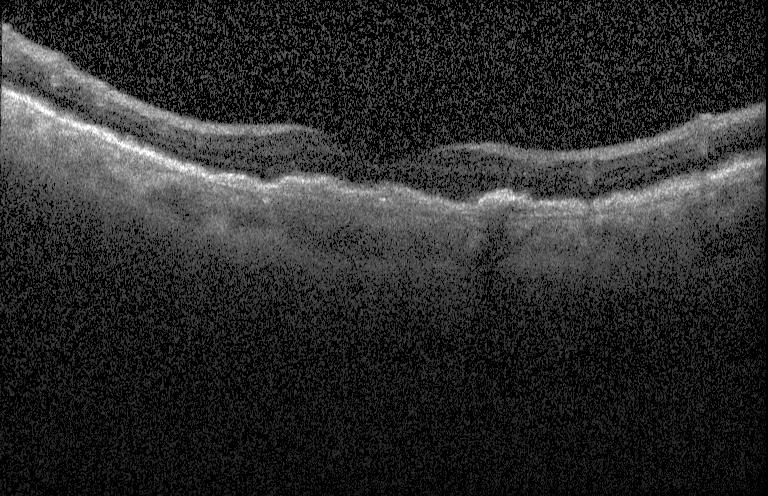 OCT finding: a choroidal neovascular membrane.